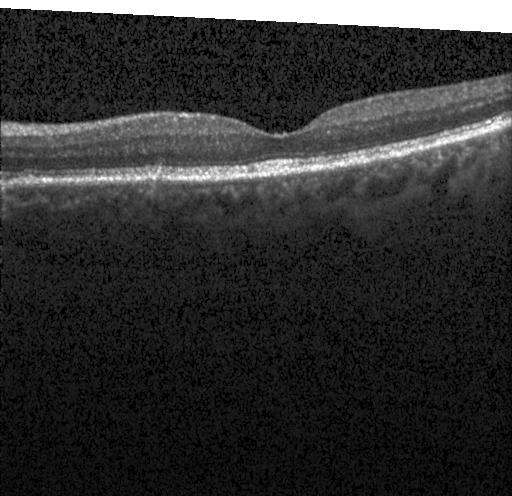 OCT B-scan.
This B-scan demonstrates neither CNV, DME, nor drusen.